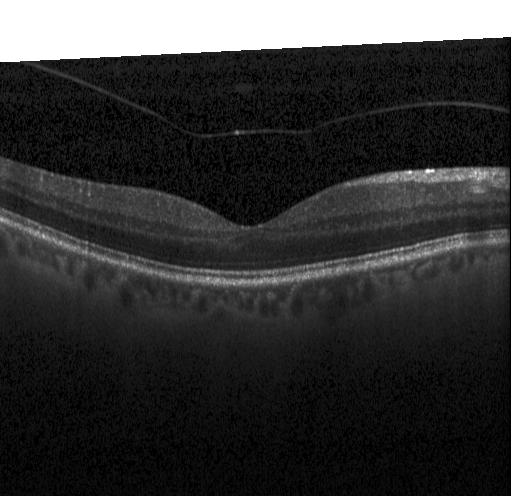
Optical coherence tomography B-scan. Dx: neither choroidal neovascularization, diabetic macular edema, nor drusen.